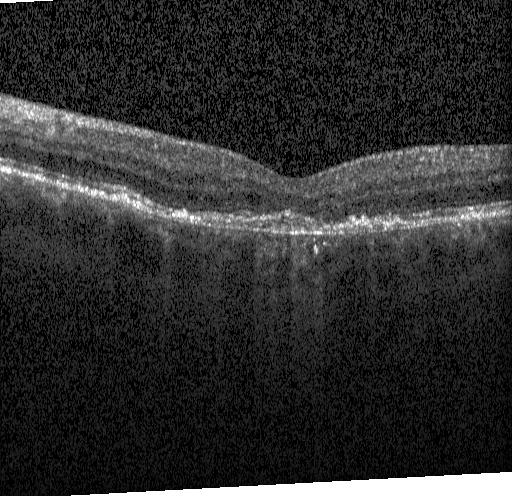
Finding: a choroidal neovascular membrane.